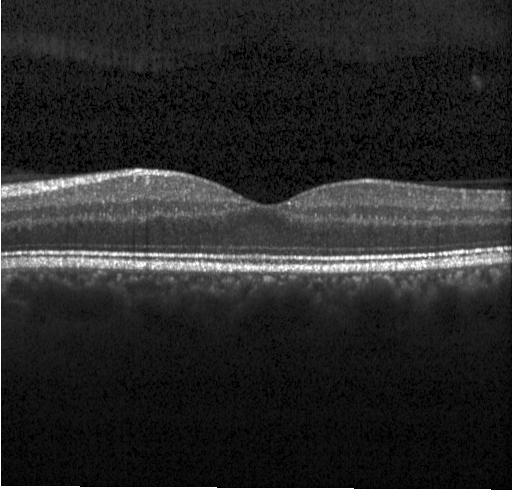

OCT scan showing no CNV, DME, or drusen.